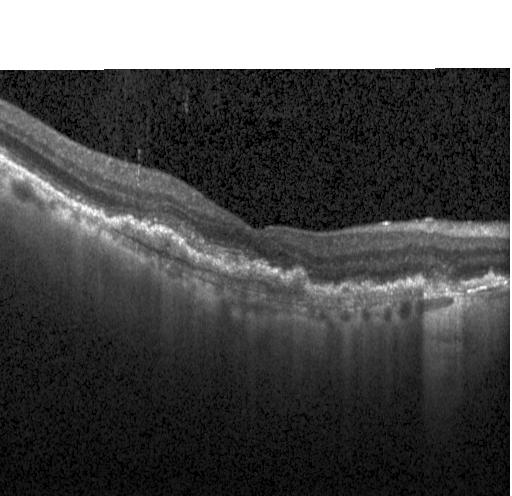
OCT B-scan. OCT finding: a choroidal neovascular membrane.